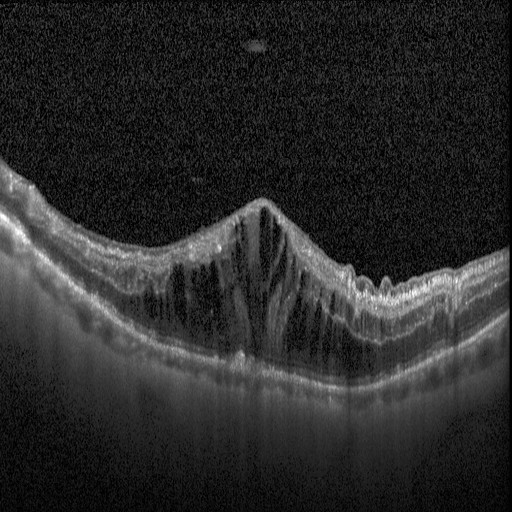 Retinal OCT B-scan. Diagnosis: diabetic macular edema.